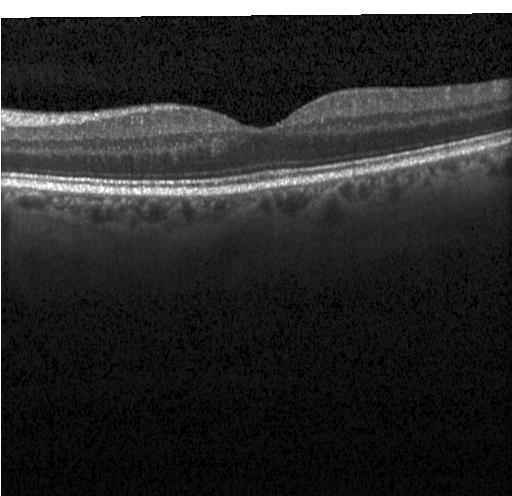 Impression: no CNV, no DME, and no drusen.